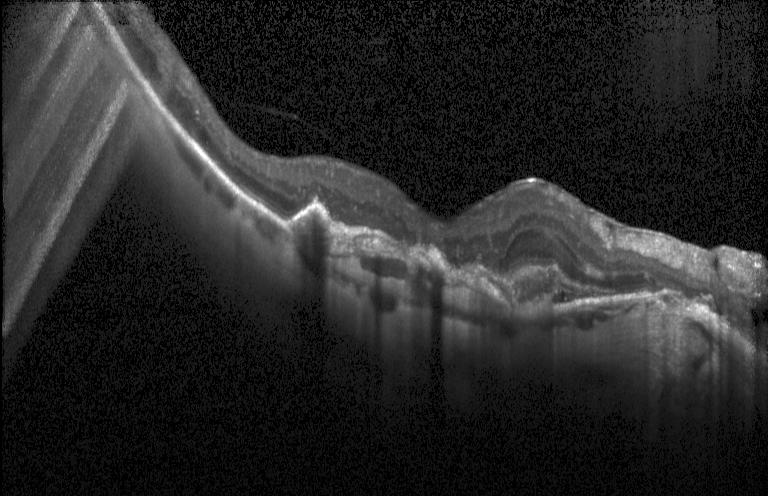 SD-OCT; retinal OCT cross-section; macular scan.
A choroidal neovascular membrane.